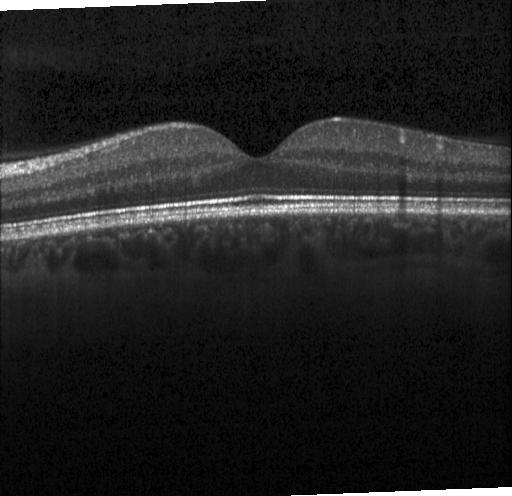
Retinal OCT cross-section.
Diagnosis: no CNV, DME, or drusen.